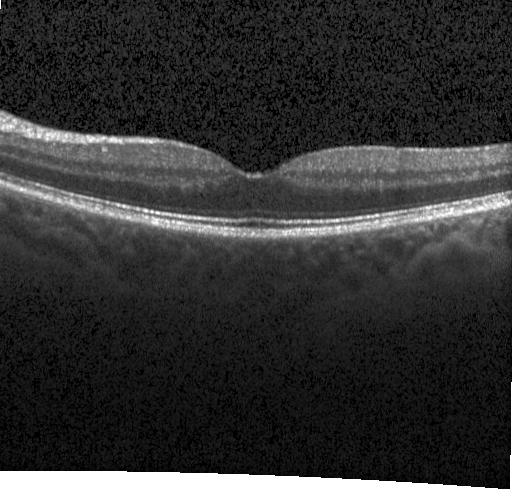

OCT B-scan — Assessment: no evidence of choroidal neovascularization, diabetic macular edema, or drusen.